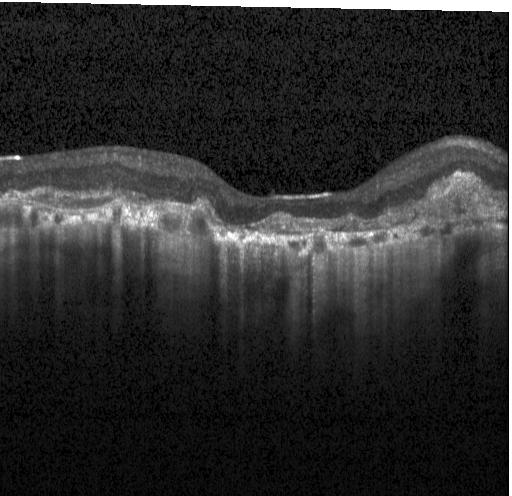 Optical coherence tomography scan · macular scan · spectral-domain OCT · Heidelberg Spectralis OCT system.
OCT finding: CNV.